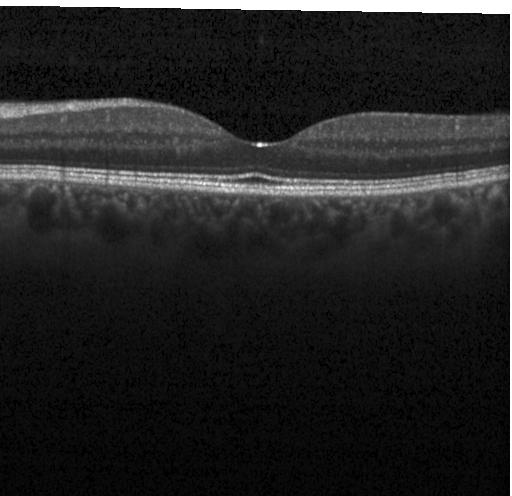 Assessment: no choroidal neovascularization, no diabetic macular edema, and no drusen.